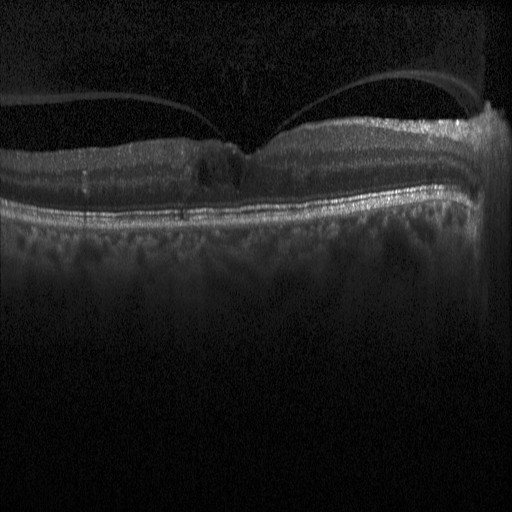
The scan shows diabetic macular edema (DME).